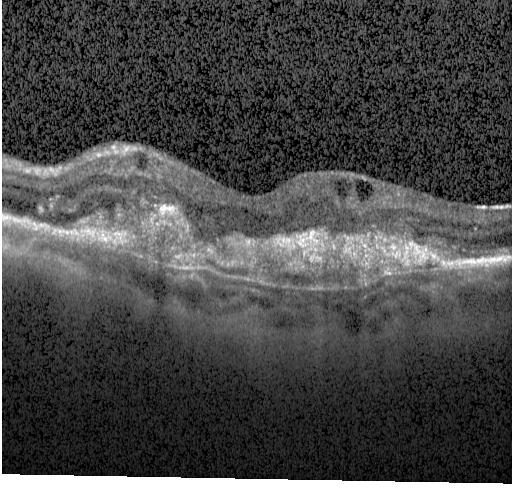 Horizontal scan through the fovea · spectral-domain optical coherence tomography · acquired on a Heidelberg Spectralis · optical coherence tomography B-scan — OCT finding: choroidal neovascularization (CNV).